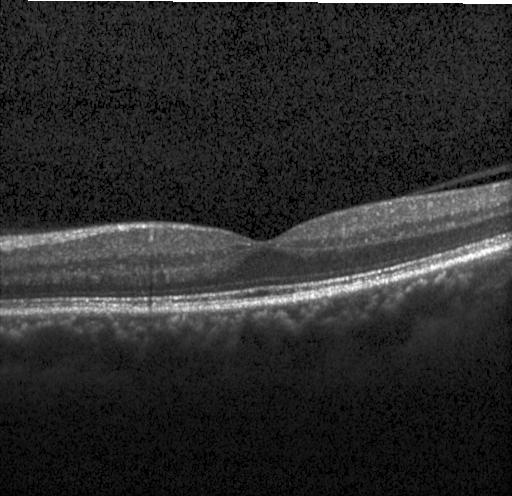

Horizontal scan through the fovea · optical coherence tomography scan · instrument: Heidelberg Spectralis · spectral-domain OCT. Impression: no CNV, DME, or drusen.